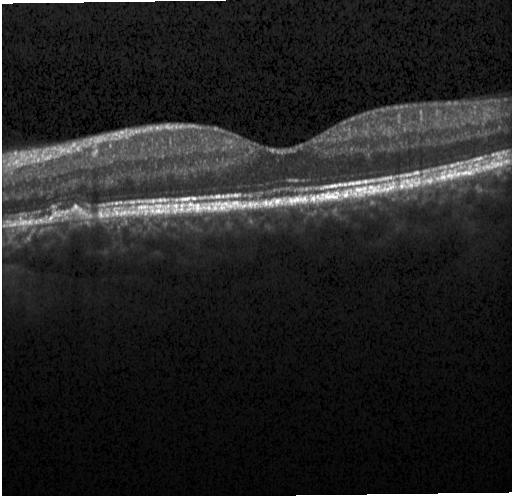

Instrument: Heidelberg Spectralis. Retinal OCT cross-section — Diagnosis: multiple drusen.